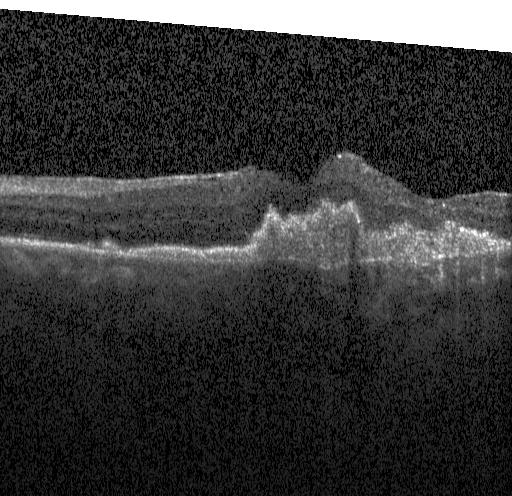 Heidelberg Spectralis, horizontal scan through the fovea, OCT B-scan, SD-OCT.
Finding: a choroidal neovascular membrane.